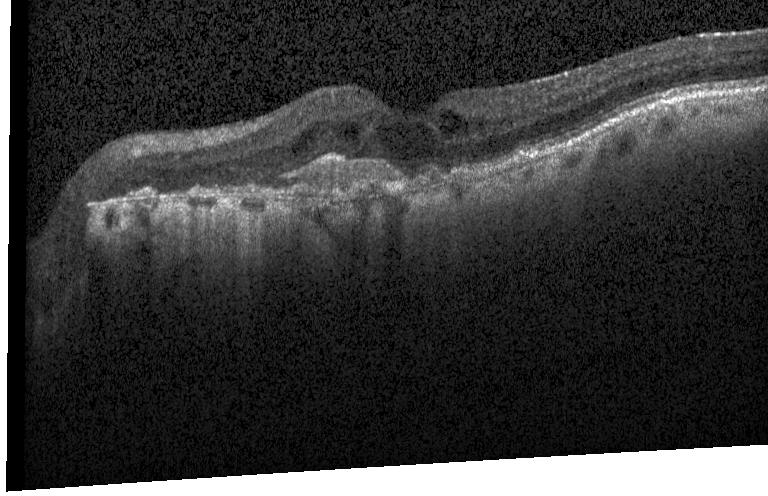
Spectral-domain optical coherence tomography · OCT line scan · instrument: Heidelberg Spectralis · centered on the fovea.
CNV.